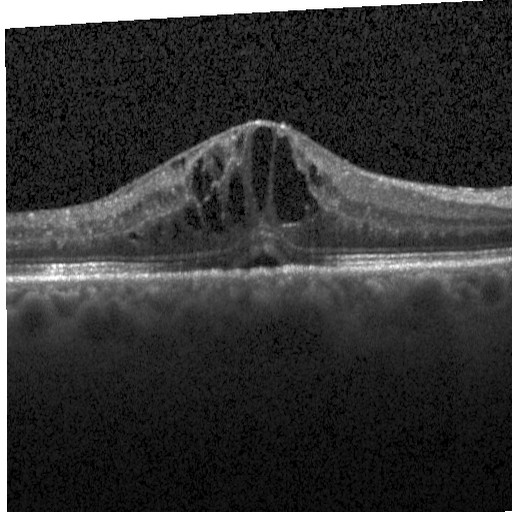
Diagnosis: diabetic macular edema (DME).